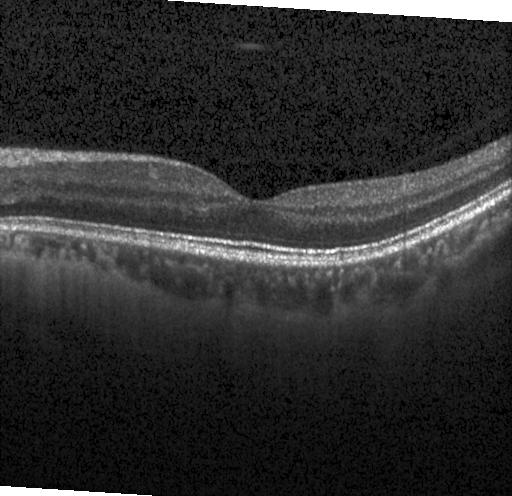
Impression: no CNV, no DME, and no drusen.